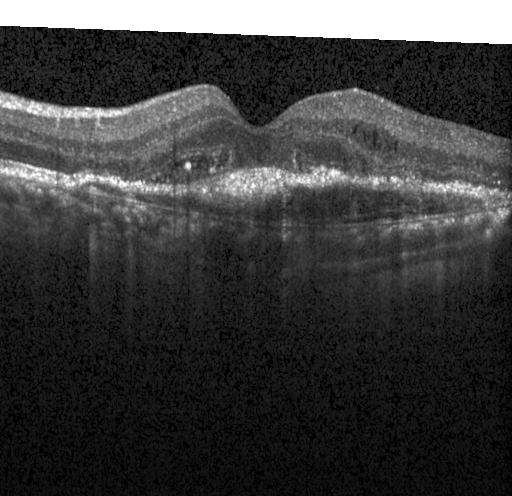
Macular scan; optical coherence tomography B-scan
The scan shows a choroidal neovascular membrane.